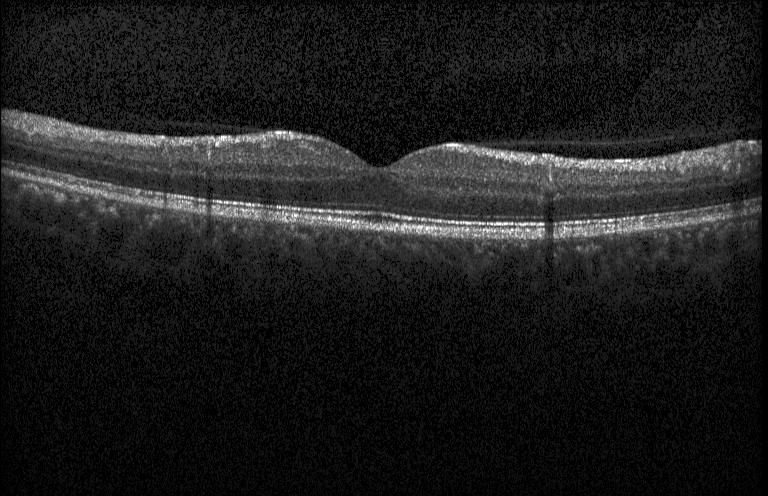 Finding: neither choroidal neovascularization, diabetic macular edema, nor drusen.